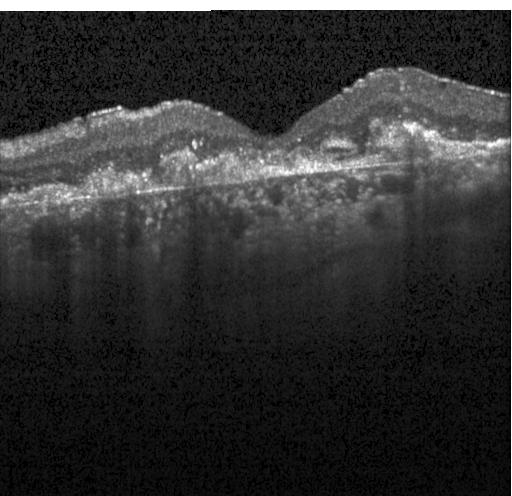
Optical coherence tomography scan · Heidelberg Spectralis OCT system · SD-OCT. Finding: CNV.